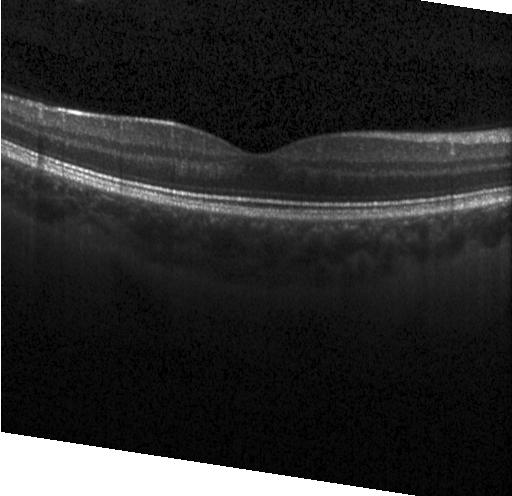

OCT scan showing neither choroidal neovascularization, diabetic macular edema, nor drusen.